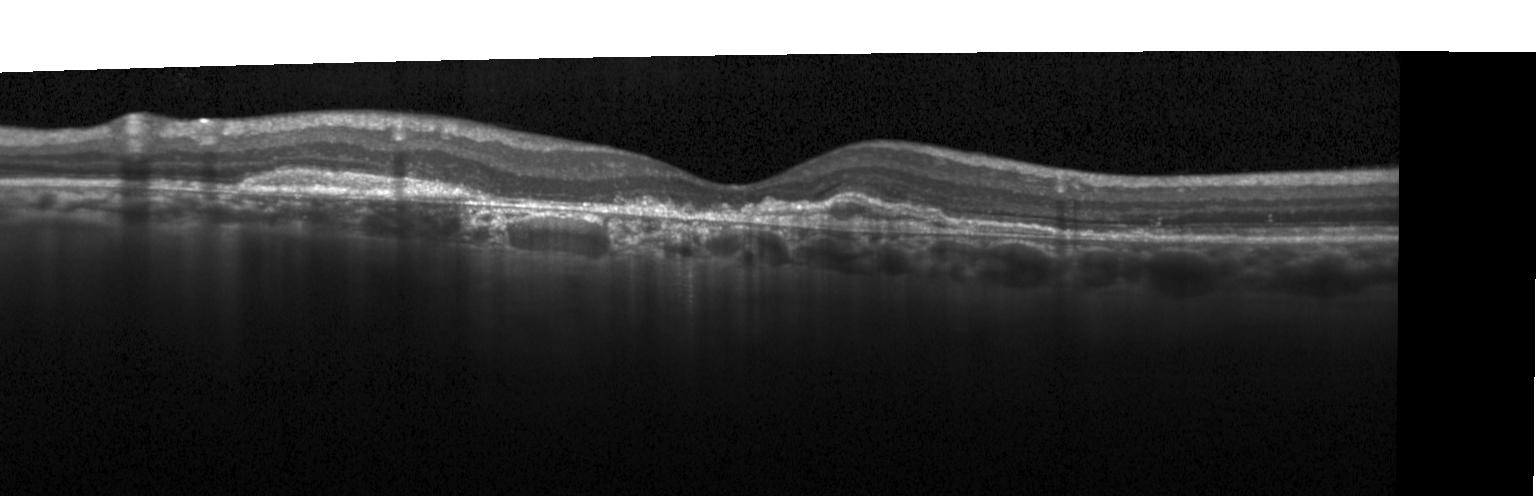

Diagnosis: CNV.